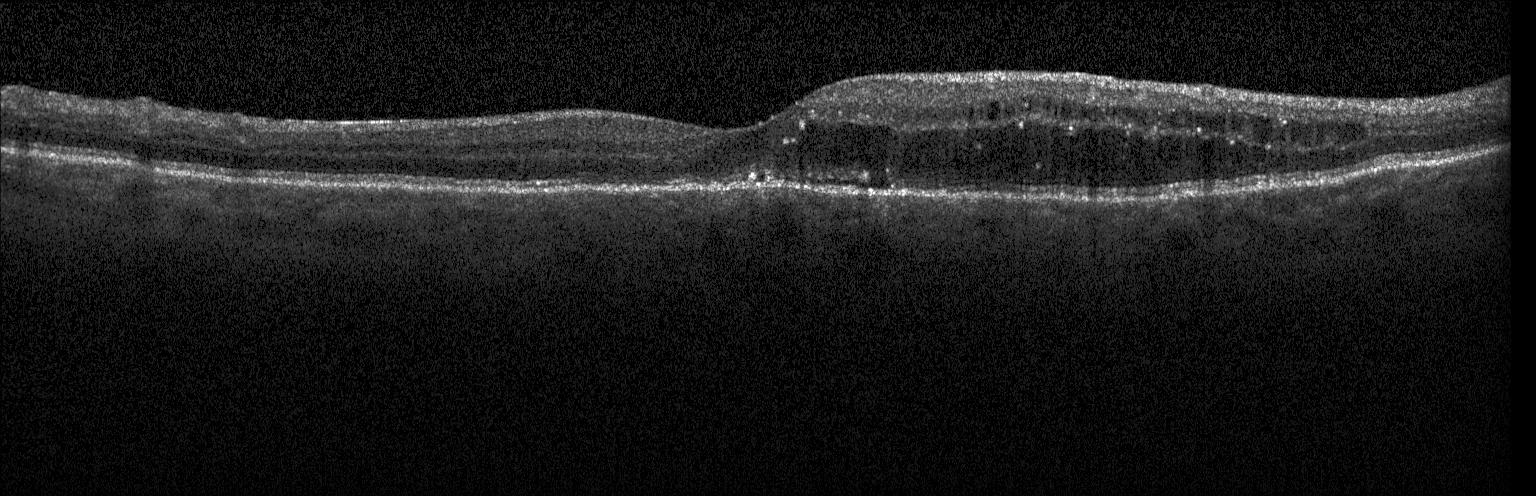

Retinal OCT cross-section.
Impression: diabetic macular edema (DME).